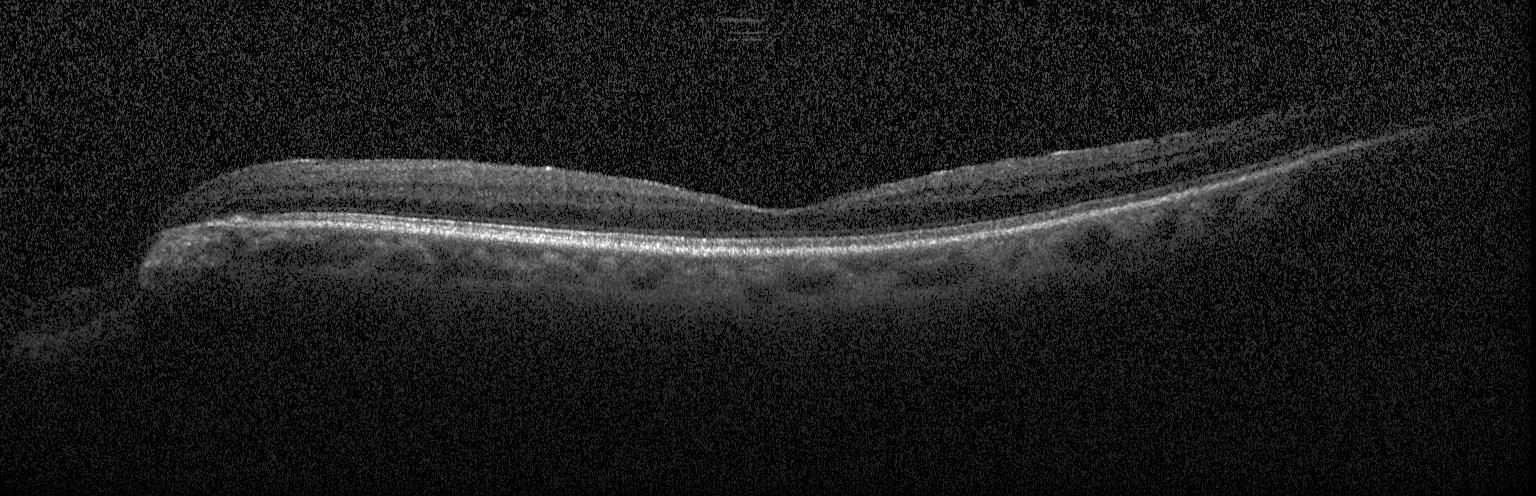
Spectral-domain OCT. Centered on the fovea. Retinal OCT B-scan — Macular OCT: neither choroidal neovascularization, diabetic macular edema, nor drusen.